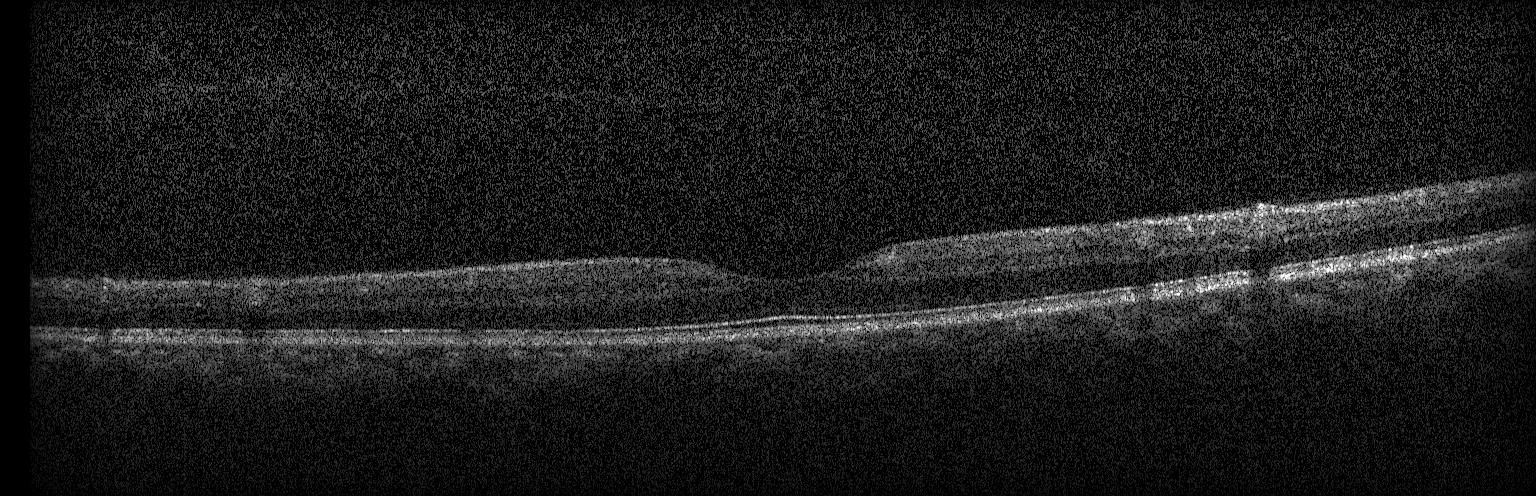

Diagnosis: no evidence of choroidal neovascularization, diabetic macular edema, or drusen.